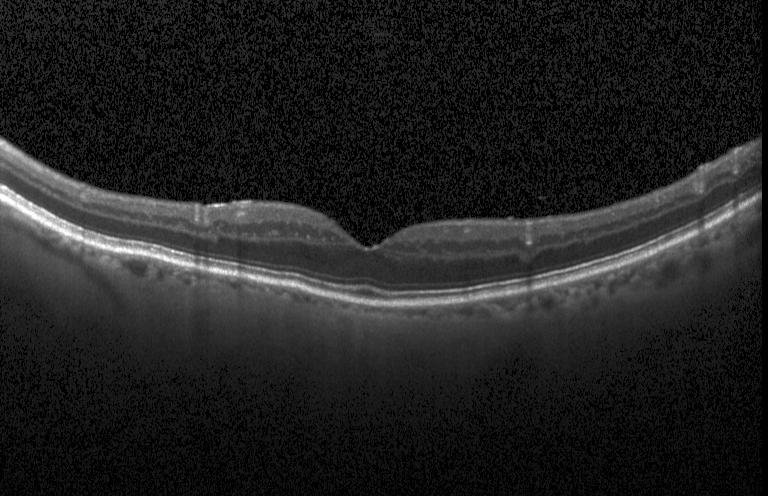

Macular OCT demonstrating no choroidal neovascularization, no diabetic macular edema, and no drusen.